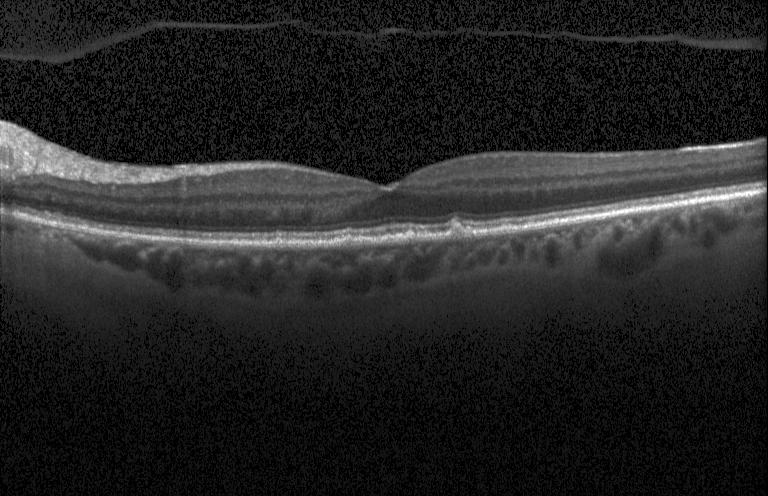
OCT scan showing drusen.